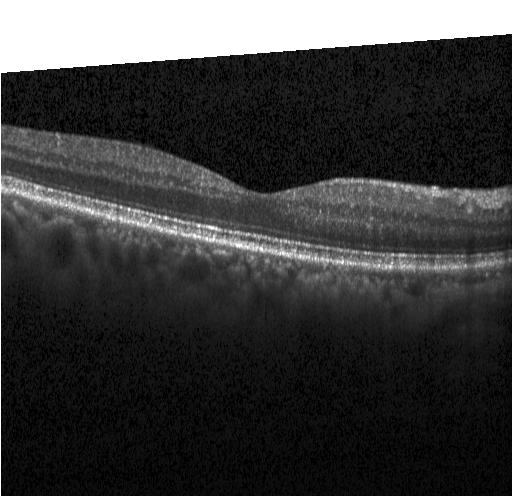

OCT line scan
Impression: no evidence of choroidal neovascularization, diabetic macular edema, or drusen.